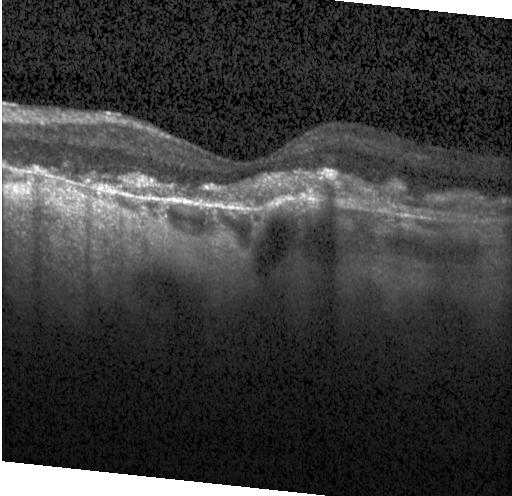
Horizontal scan through the fovea; SD-OCT; OCT B-scan
Diagnosis: choroidal neovascularization.